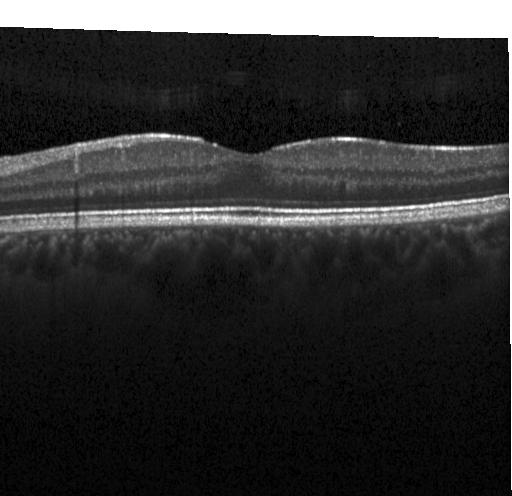
Instrument: Heidelberg Spectralis. Retinal OCT cross-section. Horizontal scan through the fovea — Diagnosis: no choroidal neovascularization, diabetic macular edema, or drusen.